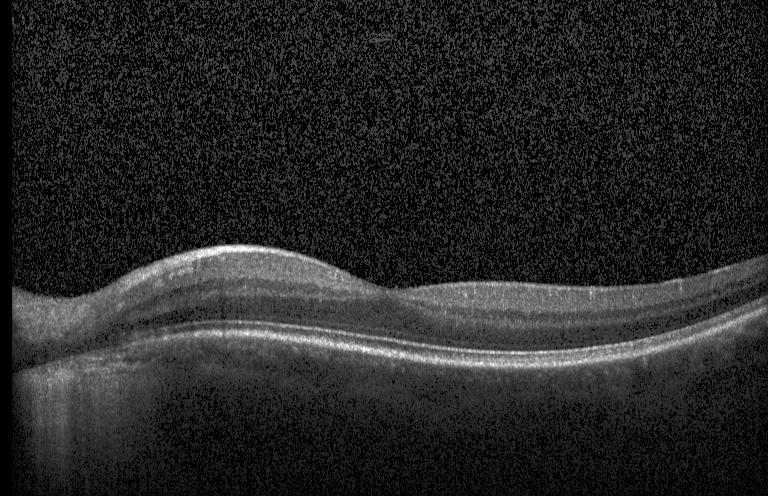

Optical coherence tomography B-scan. No choroidal neovascularization, diabetic macular edema, or drusen.